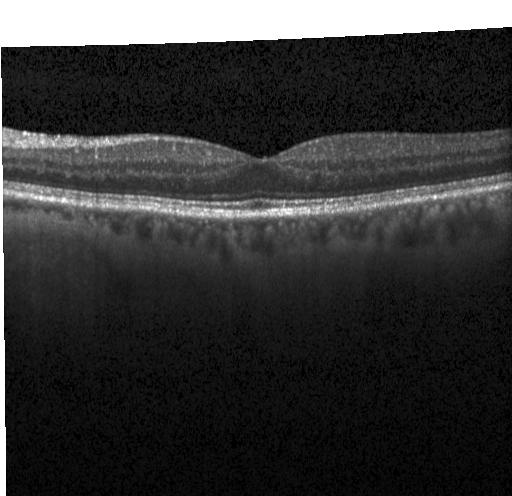 Acquired on a Heidelberg Spectralis. Centered on the fovea. Spectral-domain OCT. Retinal OCT cross-section — Finding: no evidence of choroidal neovascularization, diabetic macular edema, or drusen.